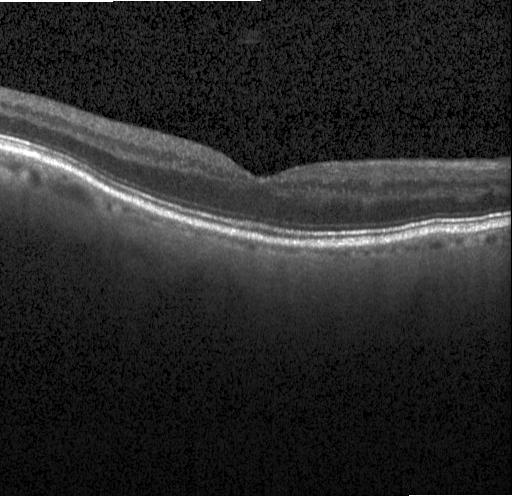
Dx: no evidence of choroidal neovascularization, diabetic macular edema, or drusen.